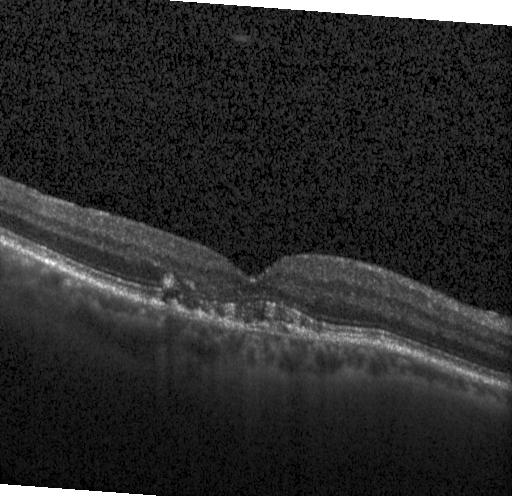
OCT scan showing a choroidal neovascular membrane.